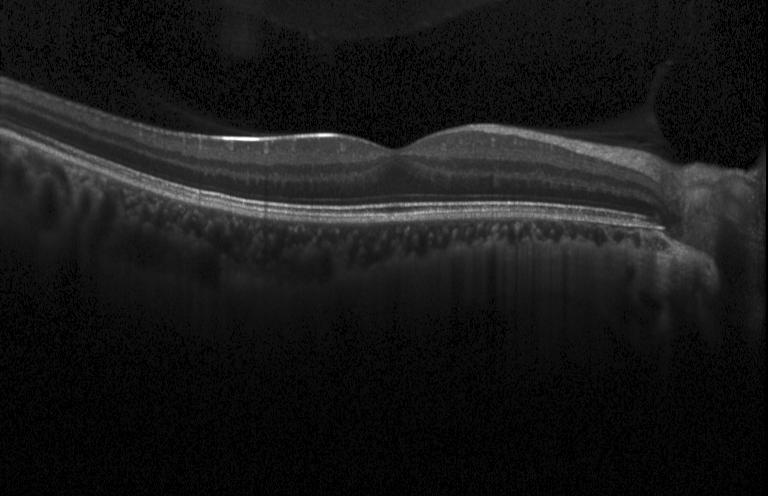

Diagnosis: no CNV, no DME, and no drusen.